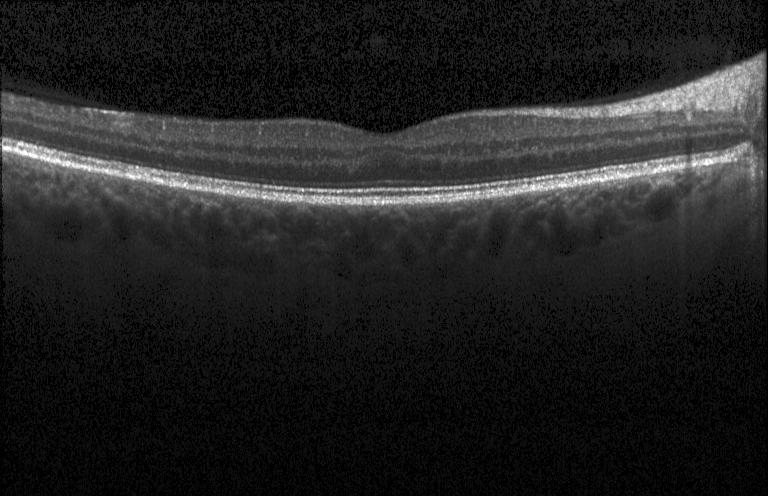 Assessment: neither CNV, DME, nor drusen.